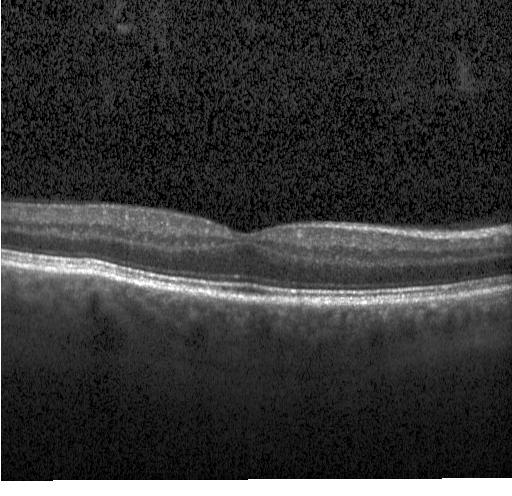
OCT scan showing no CNV, DME, or drusen.